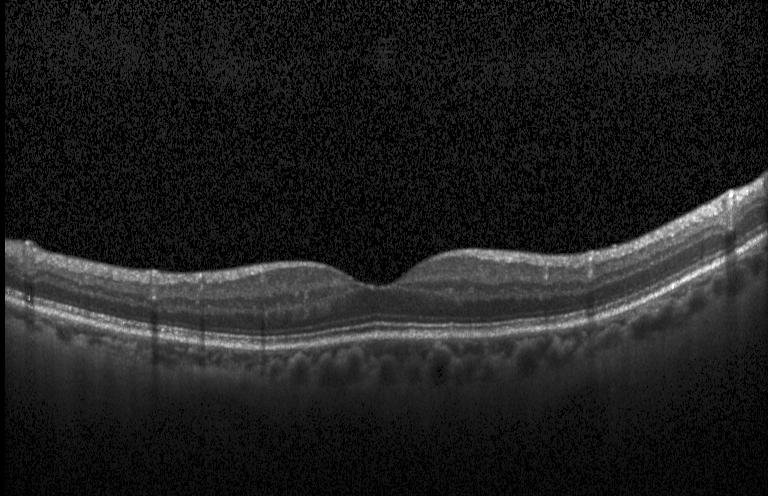
Optical coherence tomography scan, Heidelberg Spectralis — Assessment: no evidence of choroidal neovascularization, diabetic macular edema, or drusen.